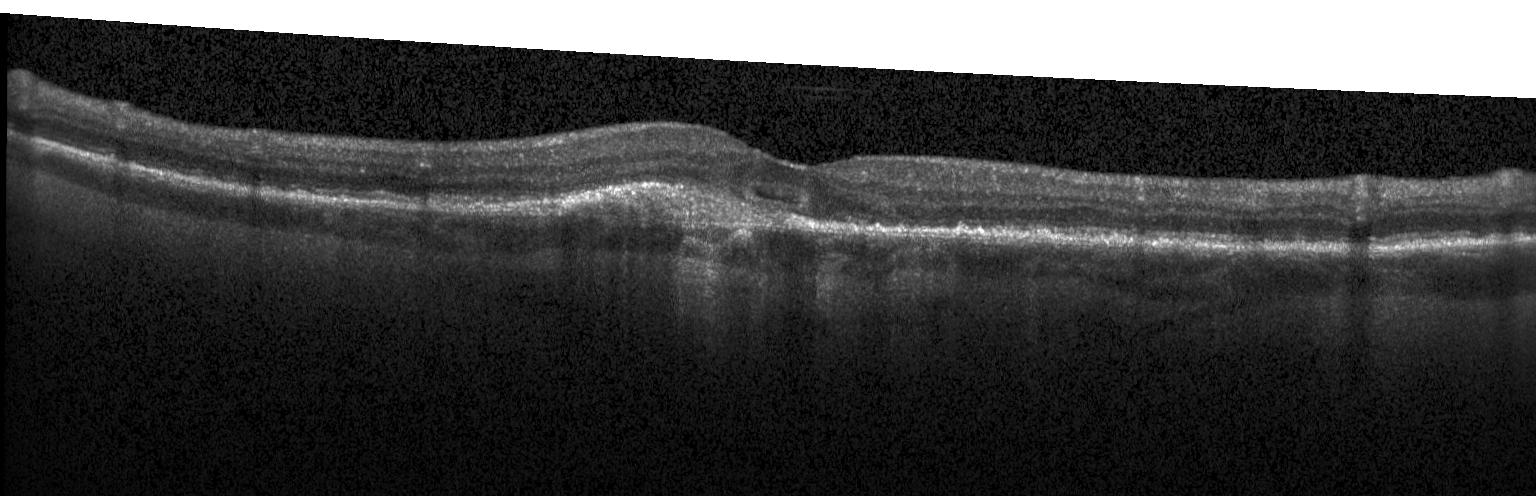 Macular OCT: a choroidal neovascular membrane.